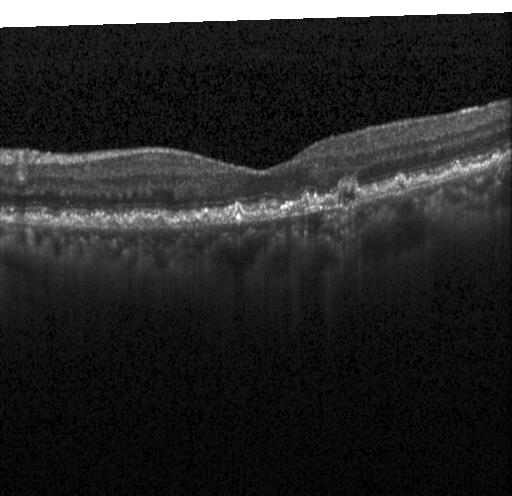

OCT B-scan
OCT finding: drusen.